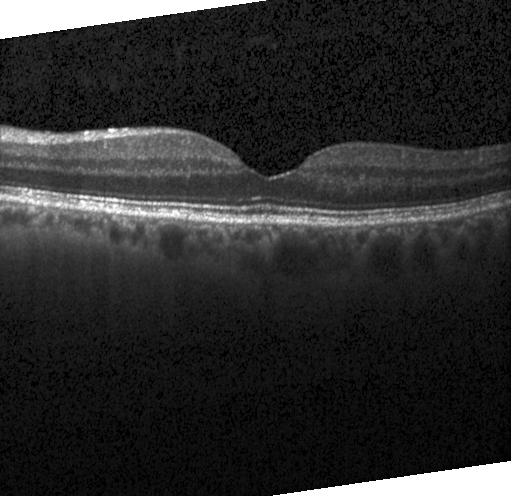

Impression: neither choroidal neovascularization, diabetic macular edema, nor drusen.